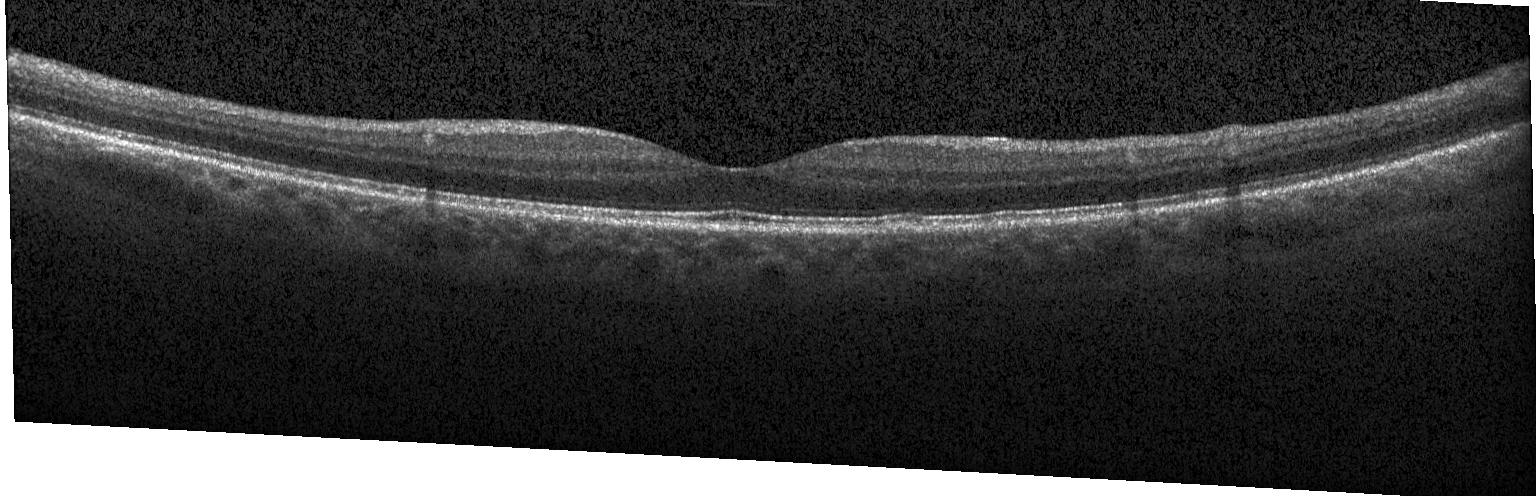
Macular scan, SD-OCT, OCT line scan, instrument: Heidelberg Spectralis
Neither CNV, DME, nor drusen.